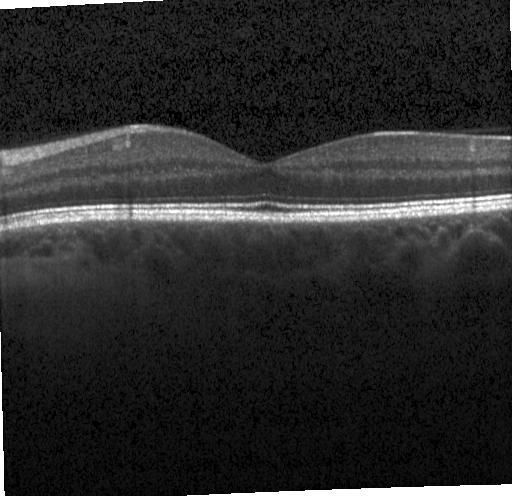

Optical coherence tomography scan. Spectral-domain OCT. Instrument: Heidelberg Spectralis — Impression: neither choroidal neovascularization, diabetic macular edema, nor drusen.